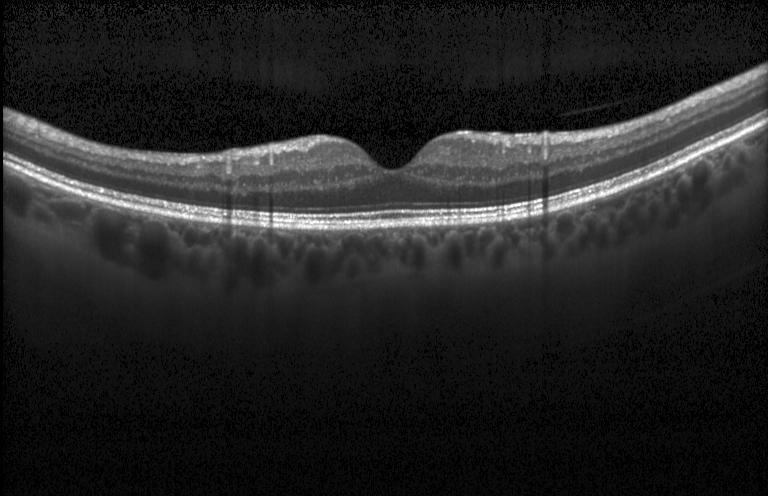
OCT line scan. Heidelberg Spectralis OCT system.
Diagnosis: no CNV, no DME, and no drusen.